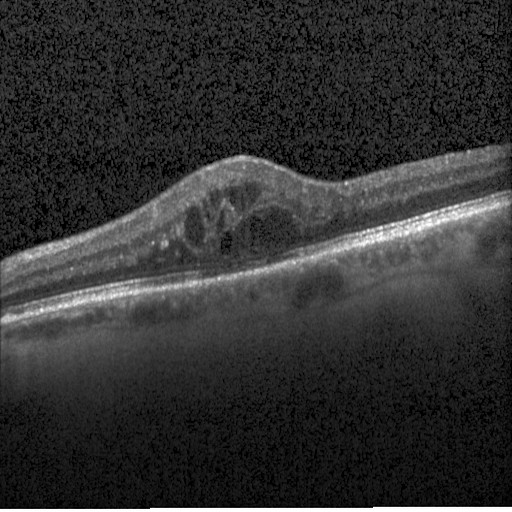 SD-OCT · horizontal scan through the fovea · Heidelberg Spectralis OCT system · OCT line scan. This B-scan demonstrates DME.